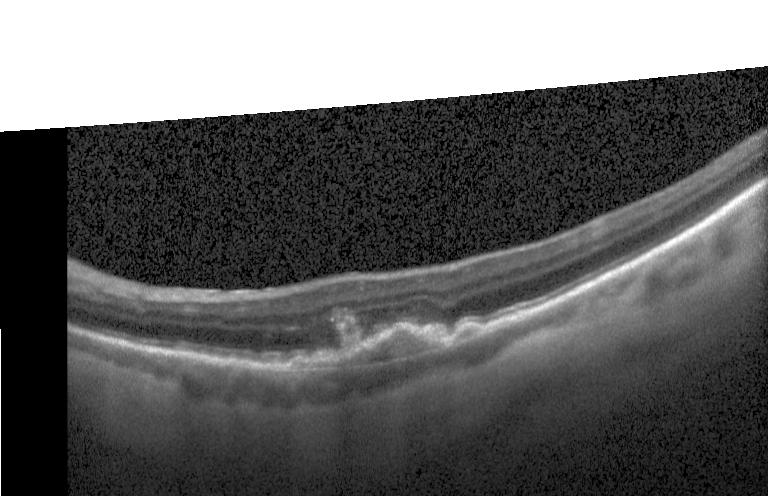

Spectral-domain OCT, optical coherence tomography B-scan, acquired on a Heidelberg Spectralis, through the macula.
Diagnosis: choroidal neovascularization.